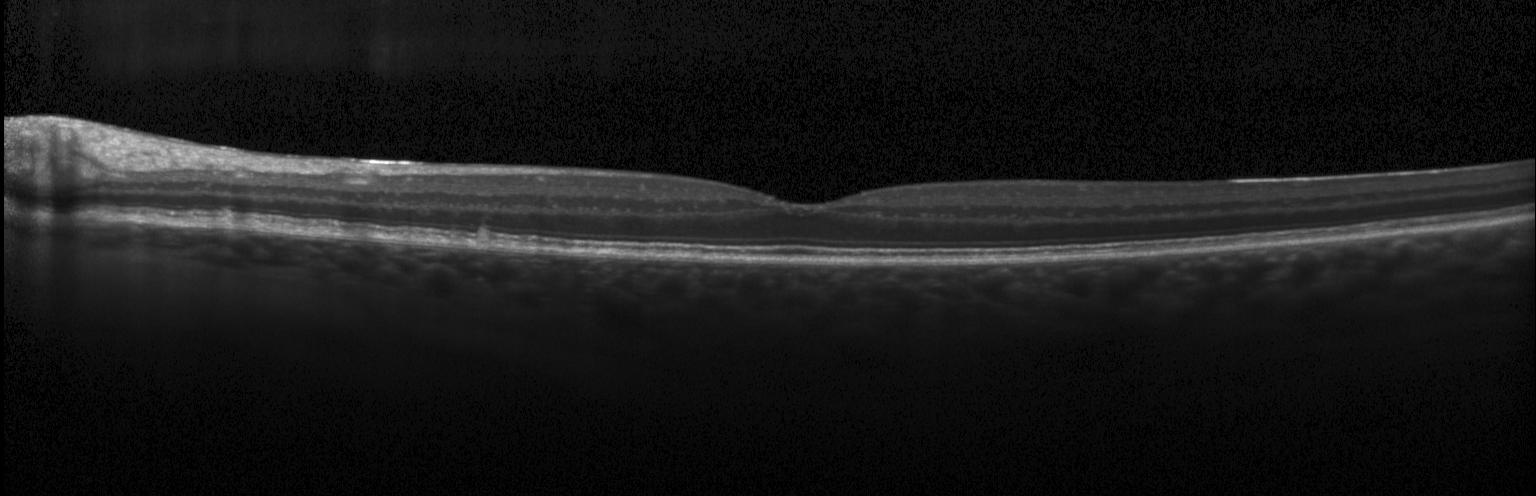

Heidelberg Spectralis · spectral-domain OCT · optical coherence tomography B-scan. This B-scan demonstrates drusen.